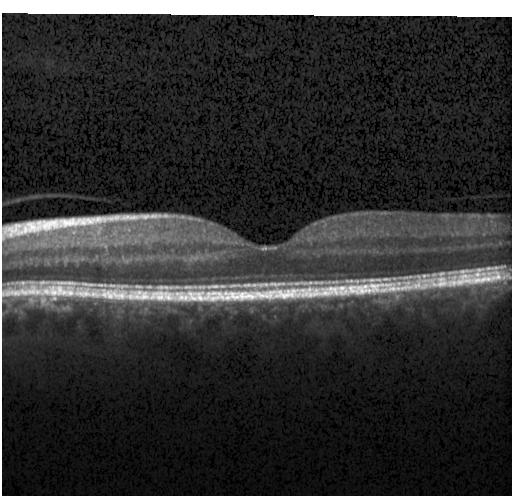

Horizontal scan through the fovea · instrument: Heidelberg Spectralis · optical coherence tomography B-scan. Dx: no evidence of choroidal neovascularization, diabetic macular edema, or drusen.